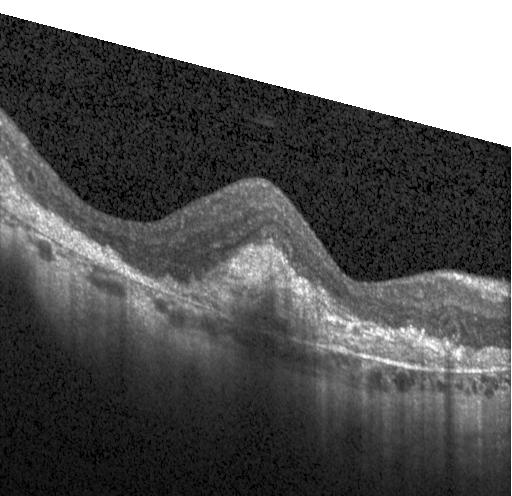
A choroidal neovascular membrane.